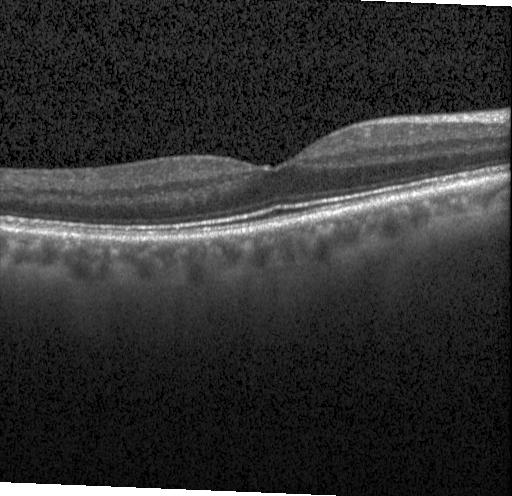 SD-OCT. Acquired on a Heidelberg Spectralis. Optical coherence tomography B-scan. Macular scan
OCT finding: no choroidal neovascularization, diabetic macular edema, or drusen.